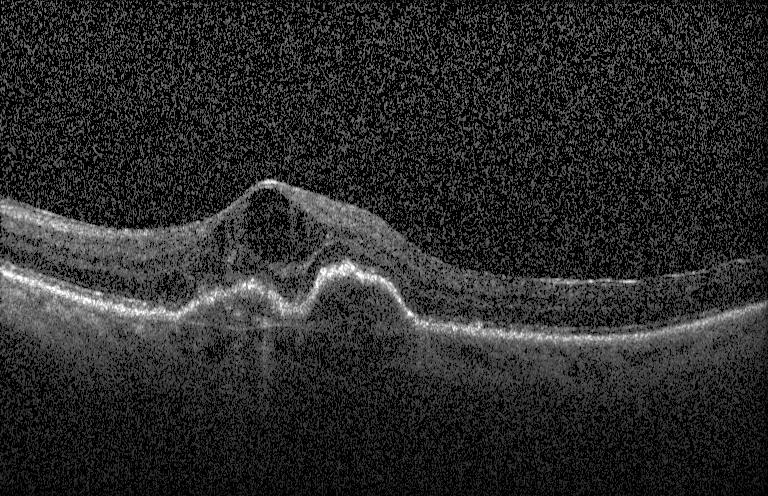 Retinal OCT B-scan. Instrument: Heidelberg Spectralis — Finding: a choroidal neovascular membrane.